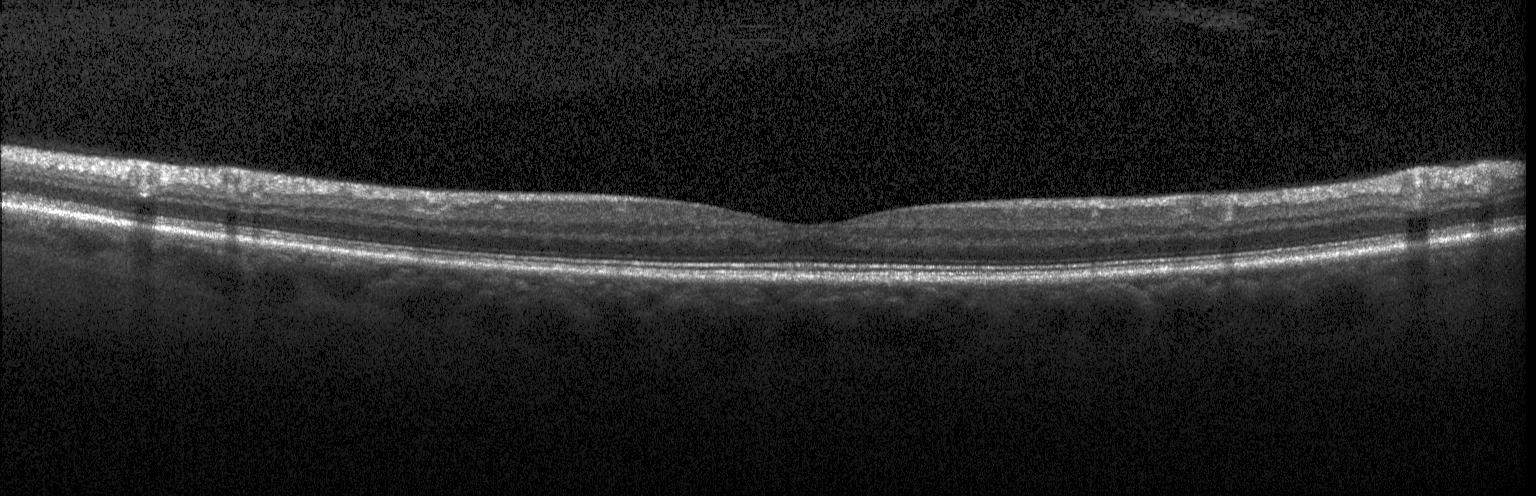
Diagnosis: neither choroidal neovascularization, diabetic macular edema, nor drusen.